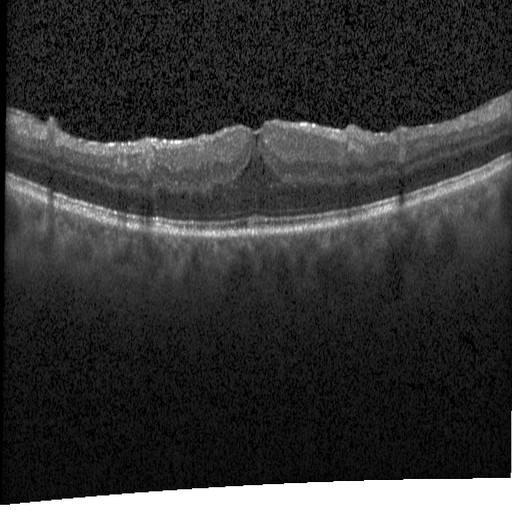
Through the macula; instrument: Heidelberg Spectralis; OCT B-scan.
This B-scan demonstrates diabetic macular edema.